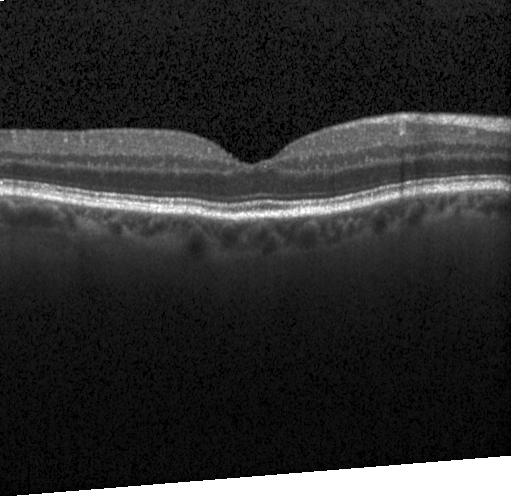 Diagnosis: neither choroidal neovascularization, diabetic macular edema, nor drusen.